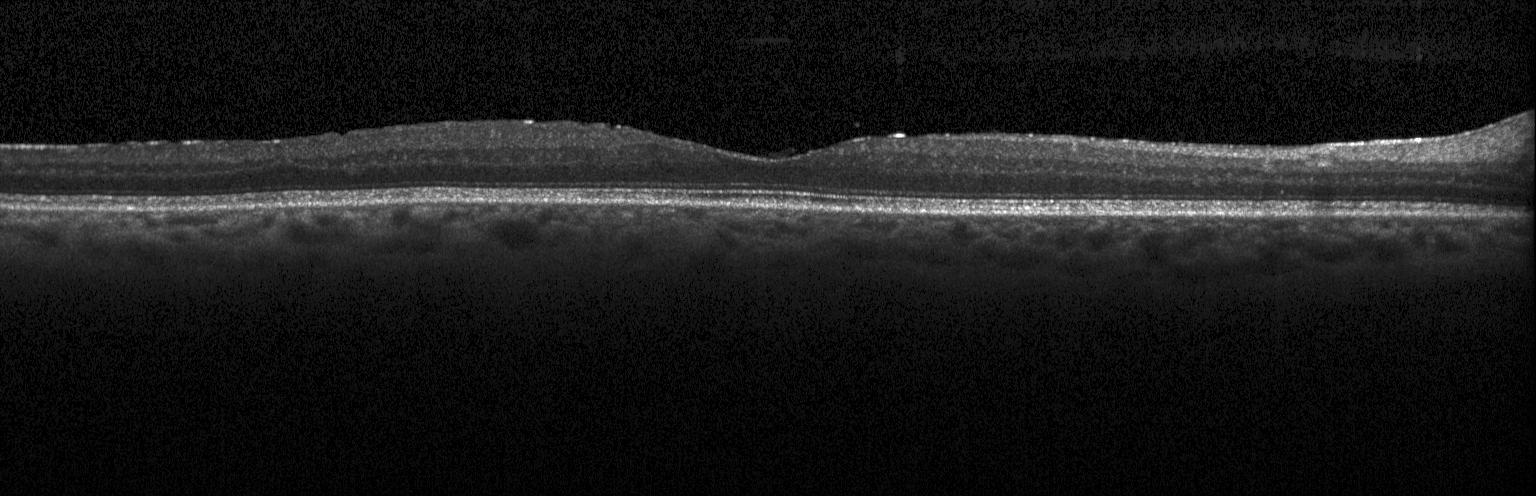 OCT line scan, acquired on a Heidelberg Spectralis, through the macula, SD-OCT — Dx: no choroidal neovascularization, diabetic macular edema, or drusen.